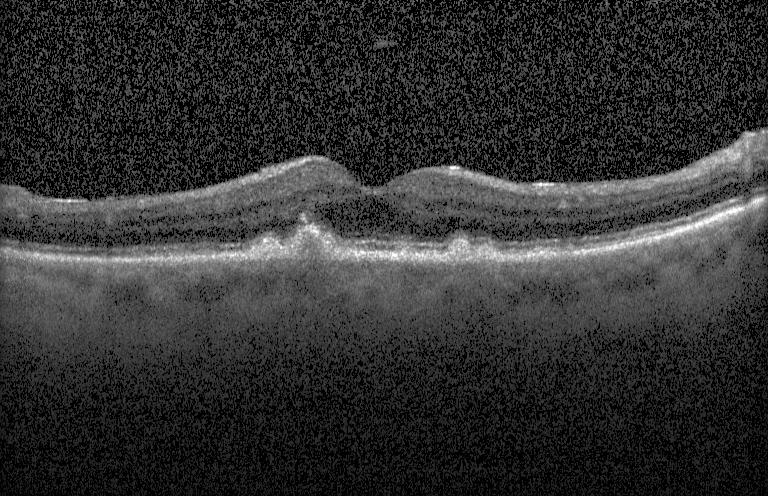

Optical coherence tomography B-scan. Instrument: Heidelberg Spectralis. Diagnosis: multiple drusen.